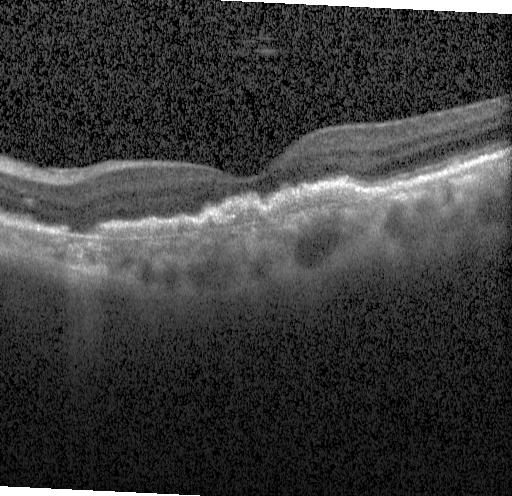
Optical coherence tomography scan. Centered on the fovea. Acquired on a Heidelberg Spectralis. Spectral-domain optical coherence tomography.
Diagnosis: a choroidal neovascular membrane.